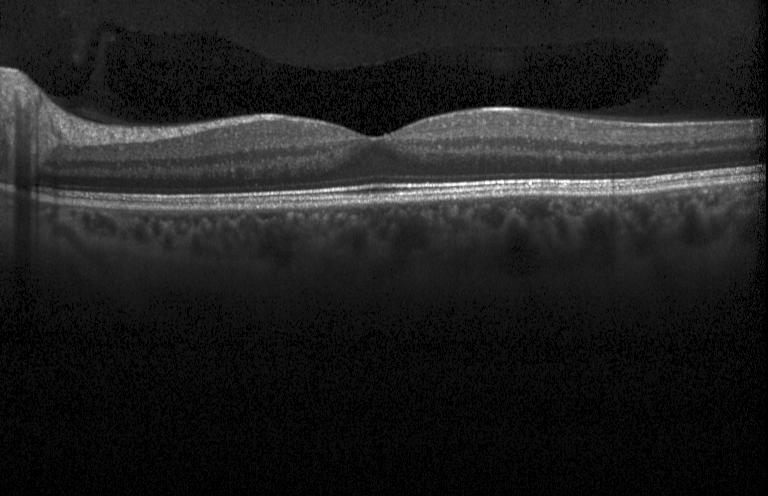 Finding: no evidence of CNV, DME, or drusen.